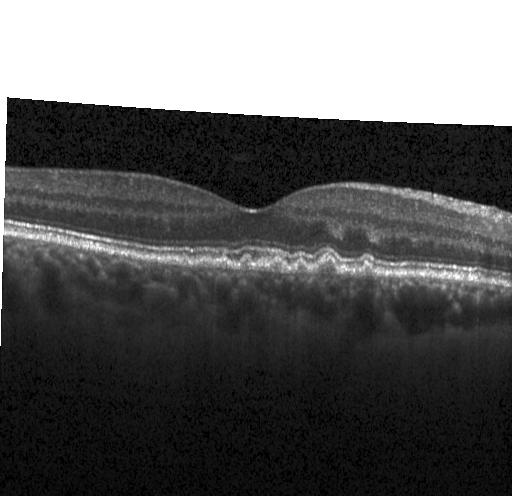

Retinal OCT B-scan, spectral-domain optical coherence tomography — Impression: multiple drusen.